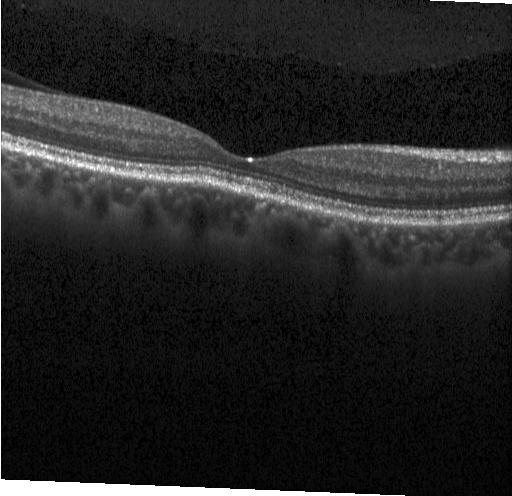

Macular OCT demonstrating no evidence of CNV, DME, or drusen.